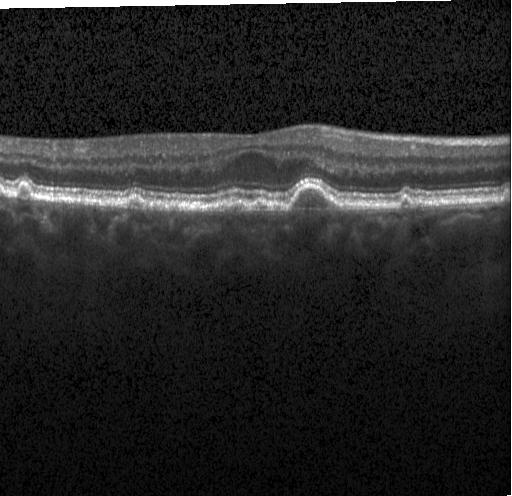

Finding: sub-RPE drusenoid deposits.